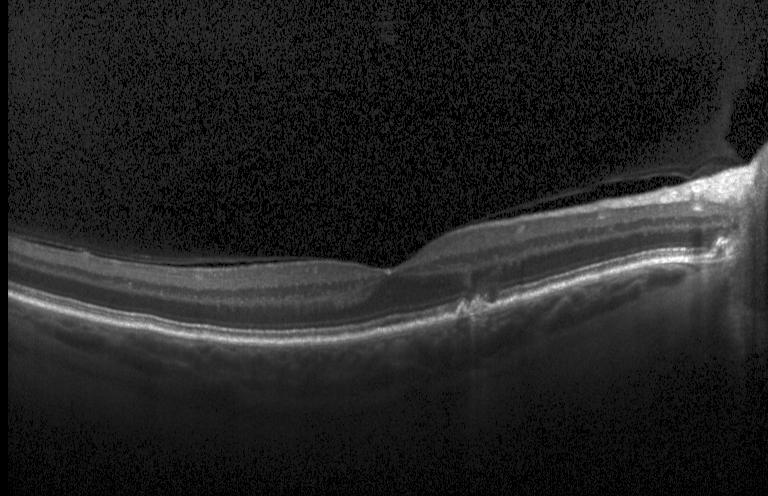 Spectral-domain OCT. Acquired on a Heidelberg Spectralis. Macular scan. Optical coherence tomography B-scan — Impression: sub-RPE drusenoid deposits.